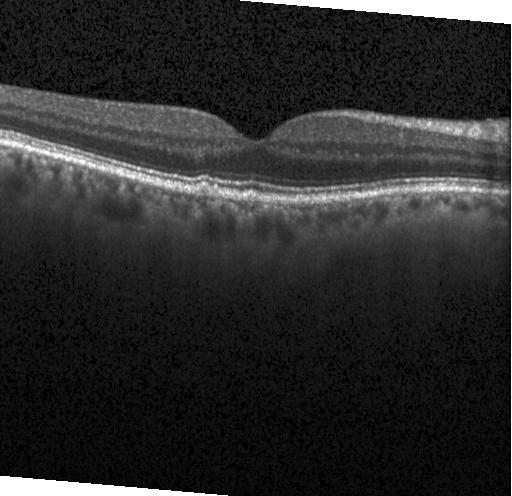
SD-OCT; through the macula; Heidelberg Spectralis OCT system; optical coherence tomography B-scan
OCT finding: sub-RPE drusenoid deposits.